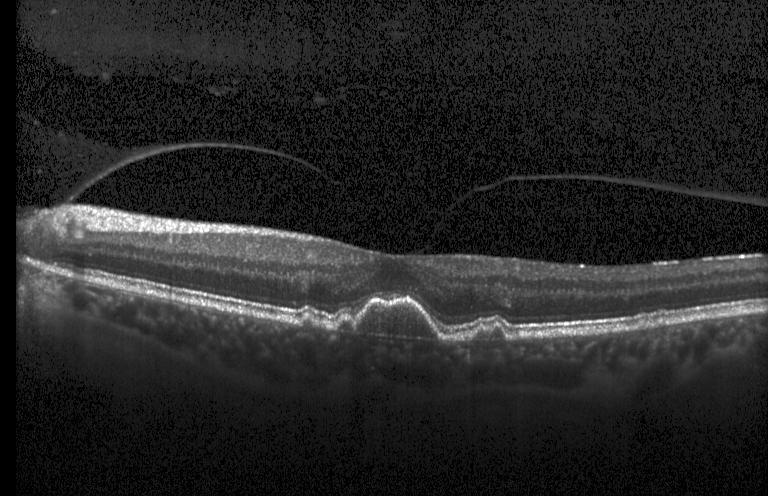 Through the macula. Retinal OCT cross-section.
Impression: multiple drusen.